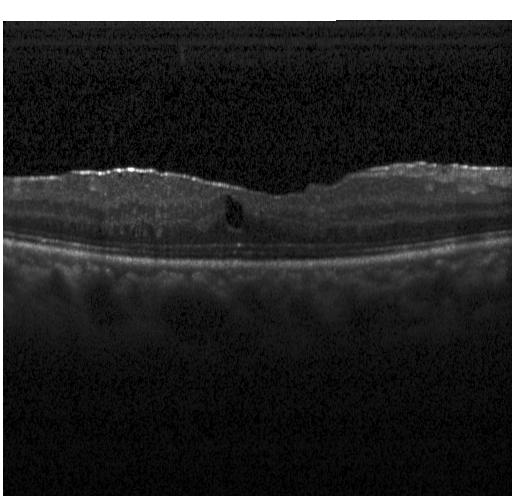

Diabetic macular edema.